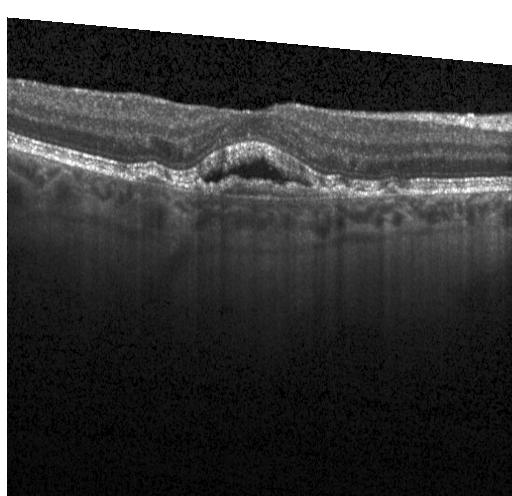

OCT scan showing a choroidal neovascular membrane.